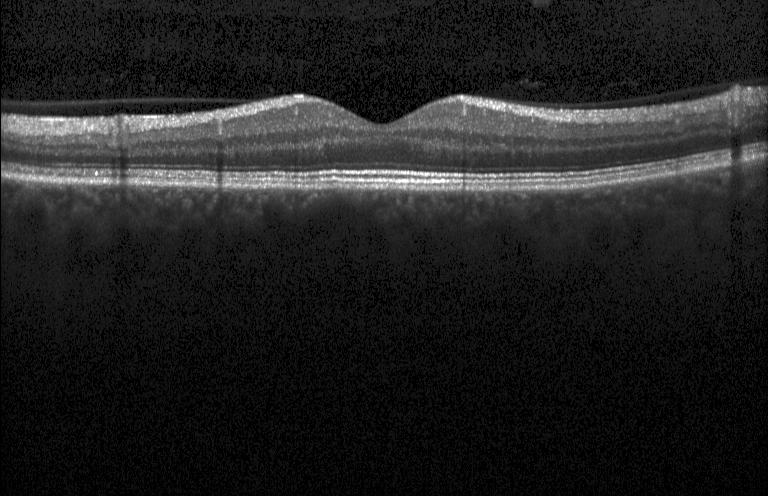 OCT B-scan showing neither CNV, DME, nor drusen.